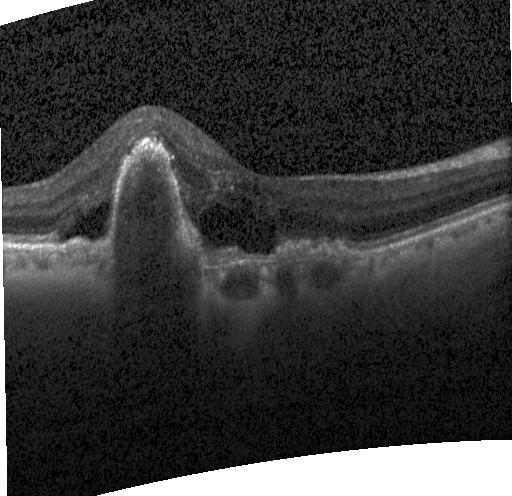
Macular OCT: a choroidal neovascular membrane.